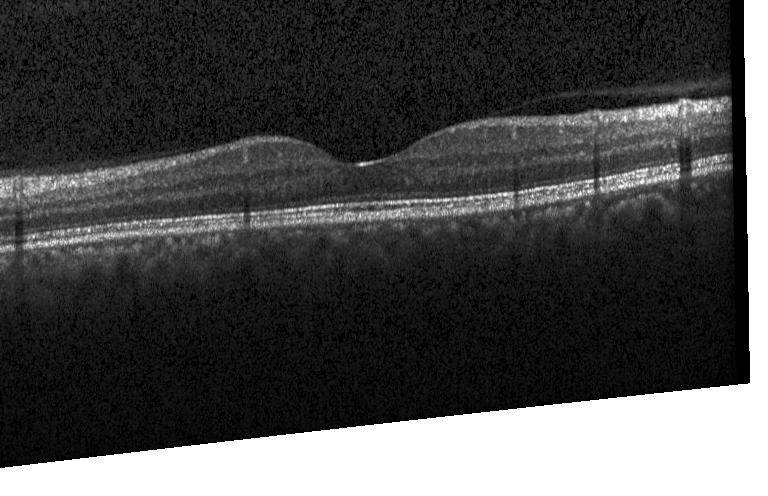
SD-OCT. Retinal OCT cross-section. Heidelberg Spectralis OCT system. Through the macula.
OCT finding: no choroidal neovascularization, no diabetic macular edema, and no drusen.